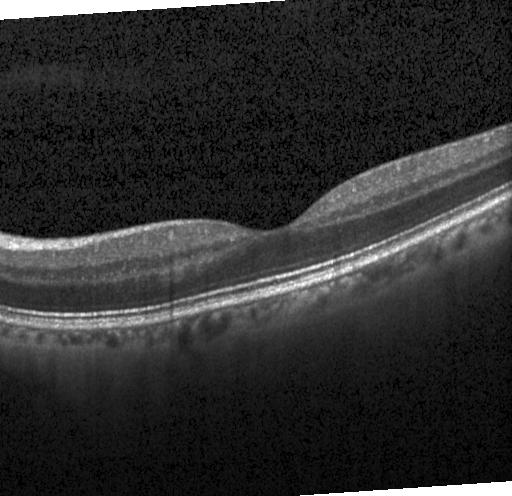 Retinal OCT B-scan · Heidelberg Spectralis OCT system · spectral-domain OCT. Diagnosis: no choroidal neovascularization, no diabetic macular edema, and no drusen.